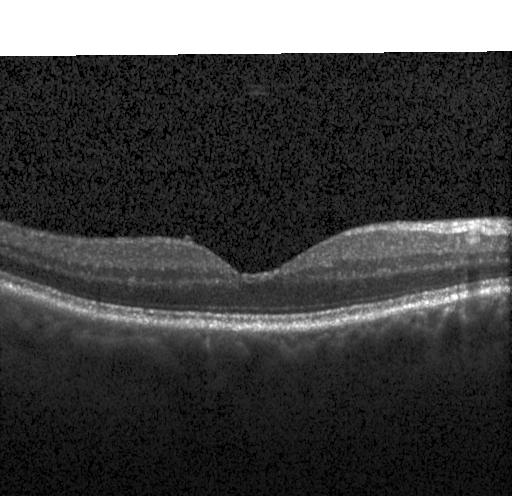 Retinal OCT cross-section showing neither CNV, DME, nor drusen.